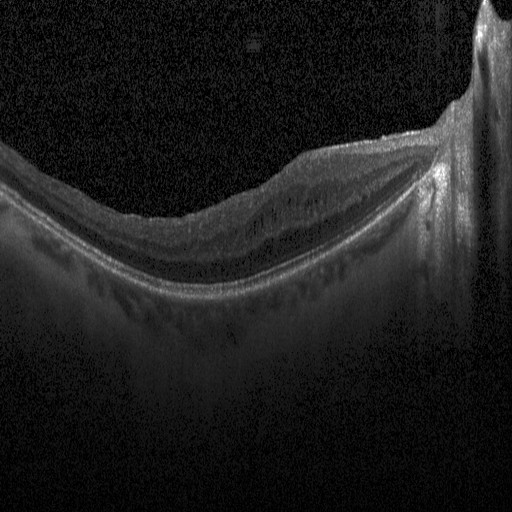
Dx: diabetic macular edema (DME).